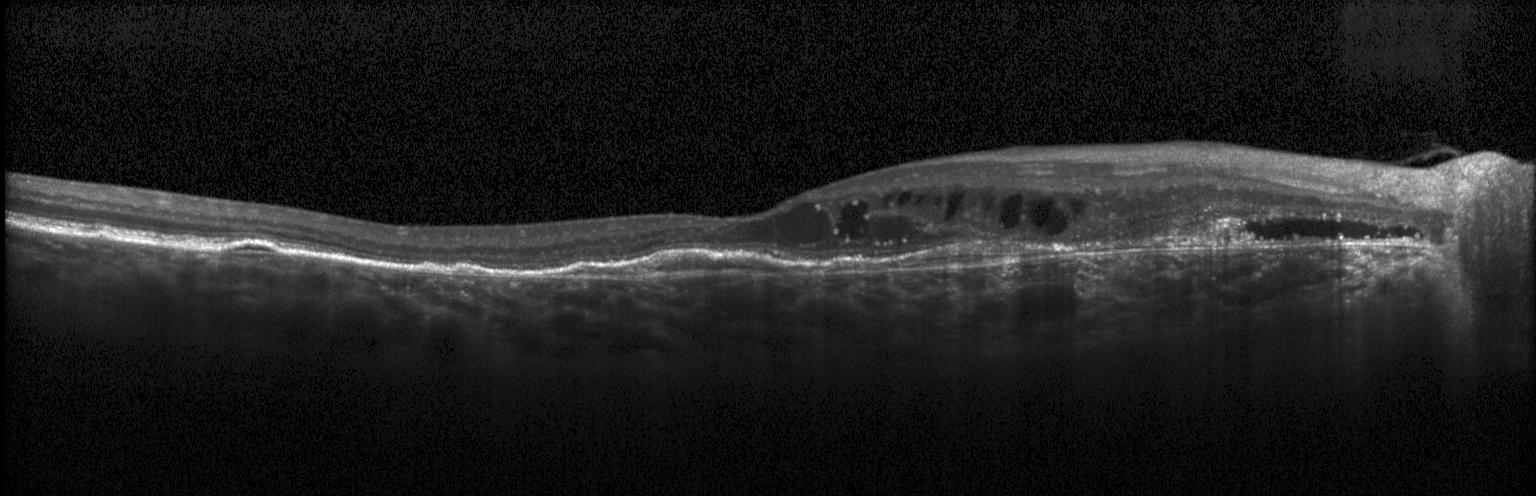 OCT finding: CNV.